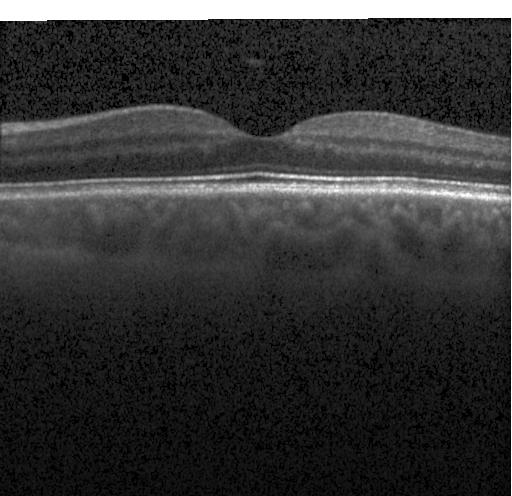 Impression: no CNV, no DME, and no drusen.